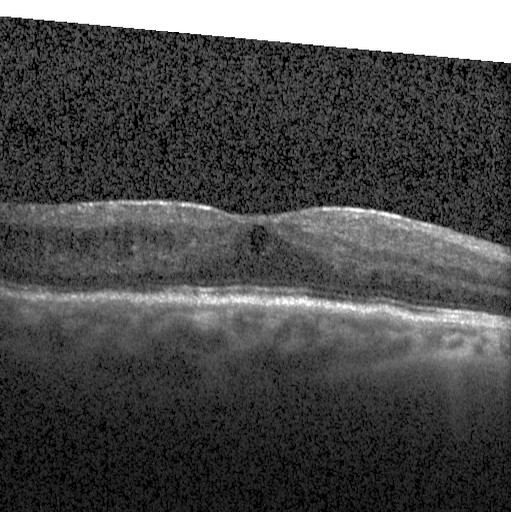 Spectral-domain OCT B-scan: diabetic macular edema (DME).